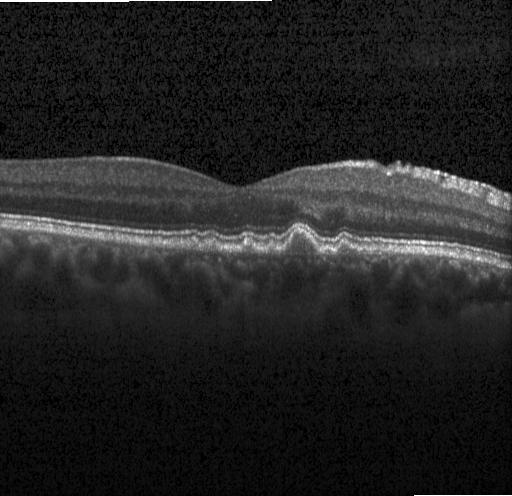
OCT line scan. Finding: multiple drusen.